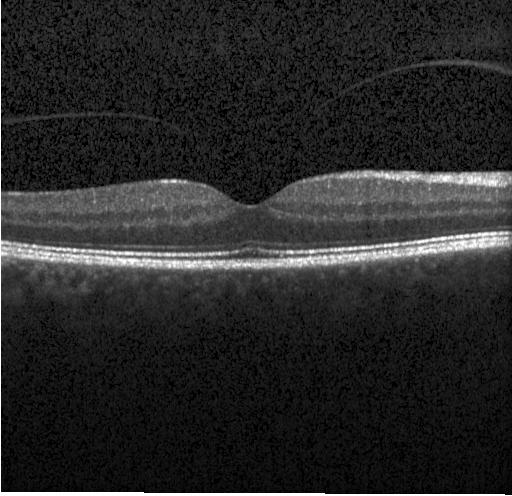 Retinal OCT B-scan. Centered on the fovea. Diagnosis: no choroidal neovascularization, diabetic macular edema, or drusen.